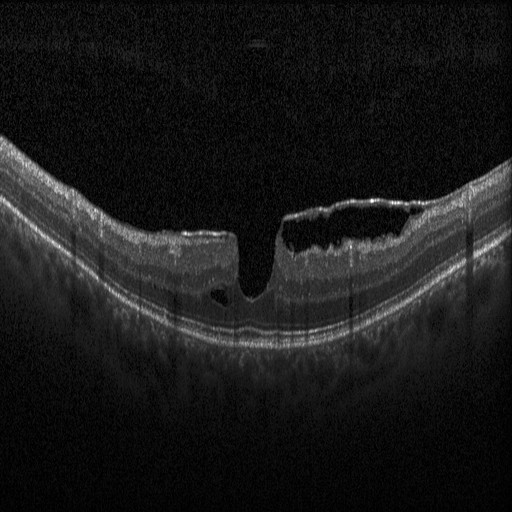
Horizontal scan through the fovea; OCT line scan; Heidelberg Spectralis
Impression: diabetic macular edema (DME).